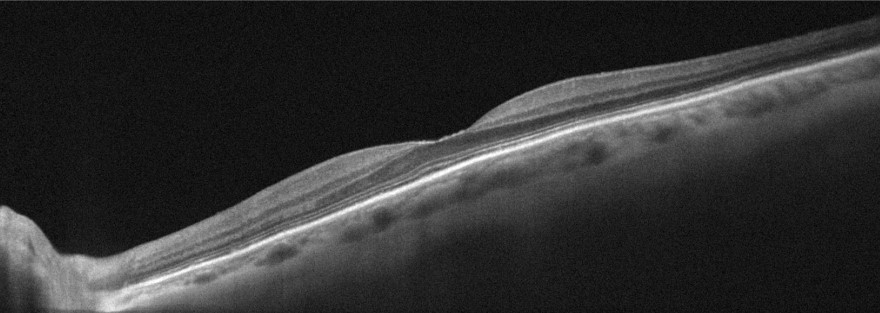

Dx: no AMD, DME, ERM, RAO, RVO, or VID.